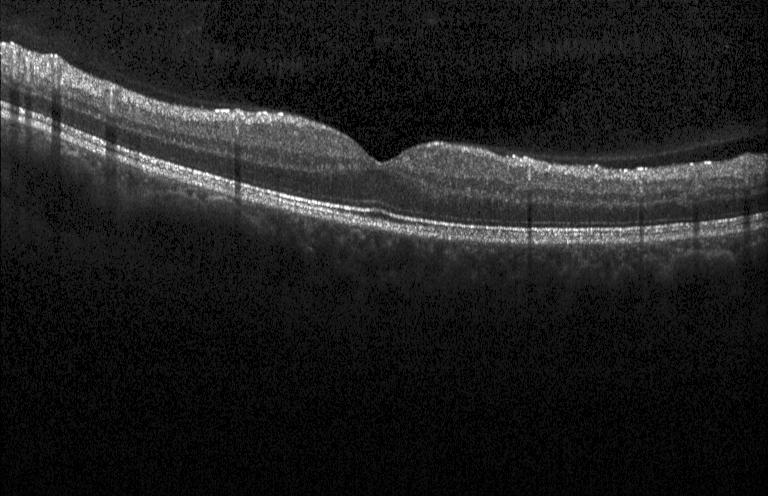
Diagnosis: no choroidal neovascularization, diabetic macular edema, or drusen.